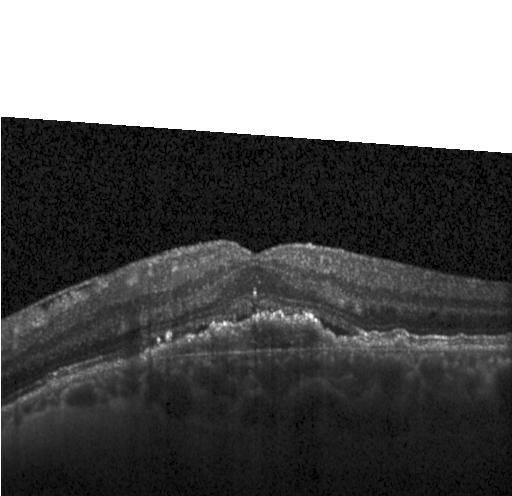

Diagnosis: a choroidal neovascular membrane.